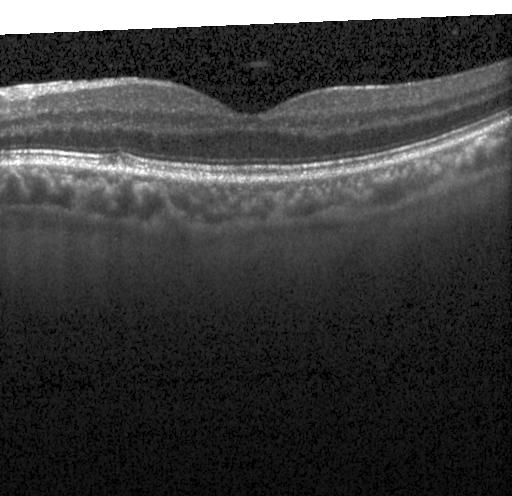

Macular scan; OCT line scan; Heidelberg Spectralis.
This B-scan demonstrates drusen.